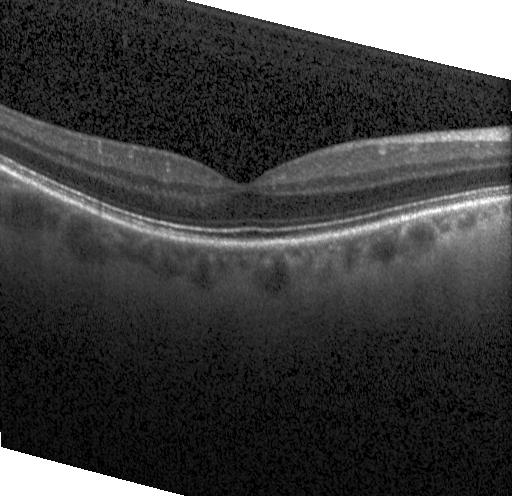
OCT finding: no choroidal neovascularization, diabetic macular edema, or drusen.